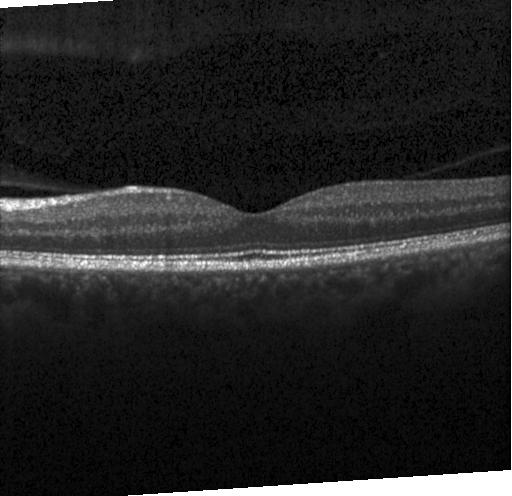

Centered on the fovea · optical coherence tomography B-scan · acquired on a Heidelberg Spectralis. Diagnosis: no evidence of choroidal neovascularization, diabetic macular edema, or drusen.